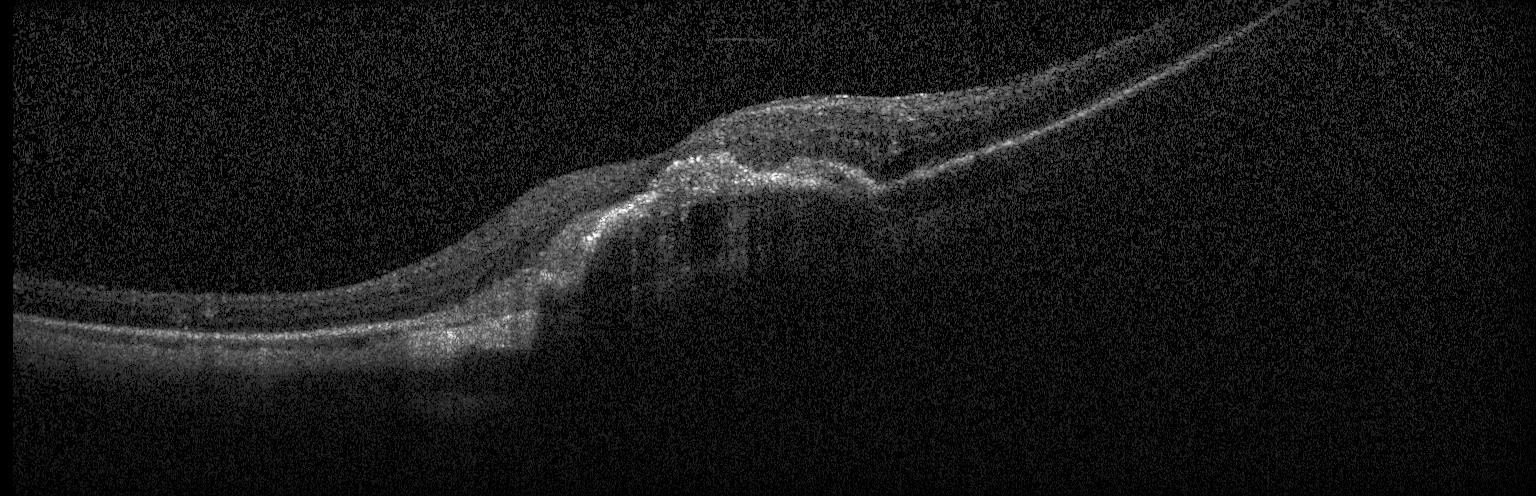

Optical coherence tomography B-scan — Diagnosis: choroidal neovascularization.